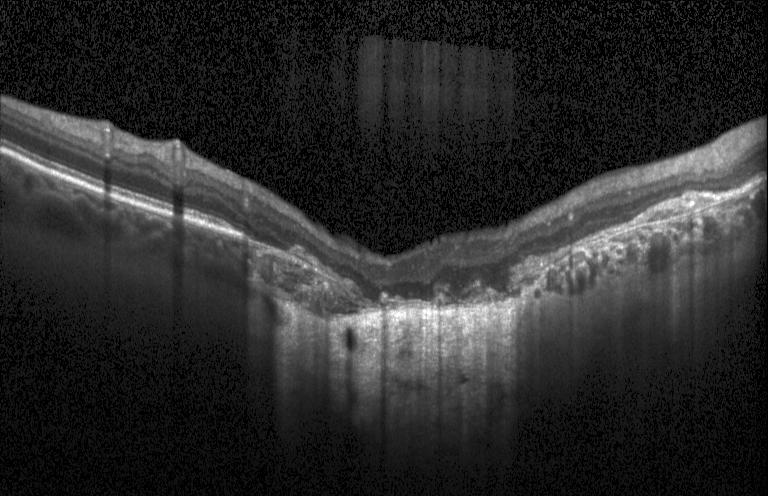
Heidelberg Spectralis, fovea-centered, OCT B-scan — Impression: a choroidal neovascular membrane.